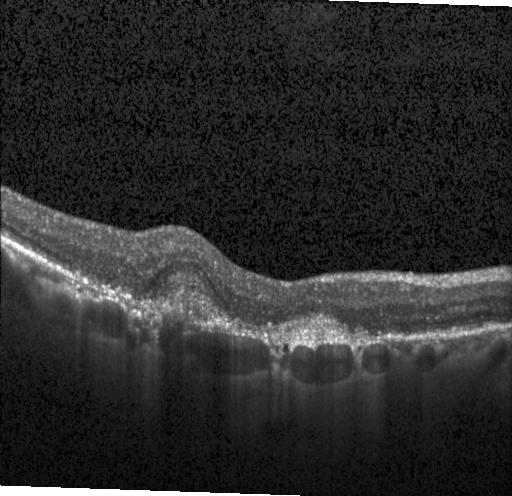

Instrument: Heidelberg Spectralis, OCT B-scan, macular scan, spectral-domain OCT.
This B-scan demonstrates choroidal neovascularization.